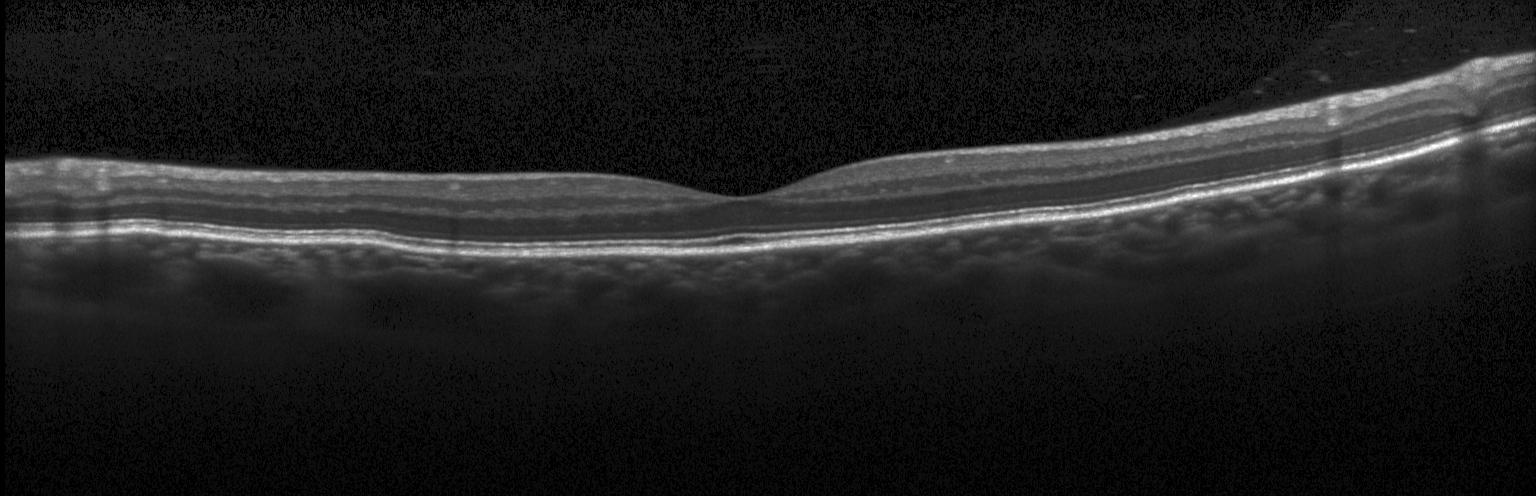 Instrument: Heidelberg Spectralis. Retinal OCT B-scan. Spectral-domain optical coherence tomography
Impression: no choroidal neovascularization, no diabetic macular edema, and no drusen.